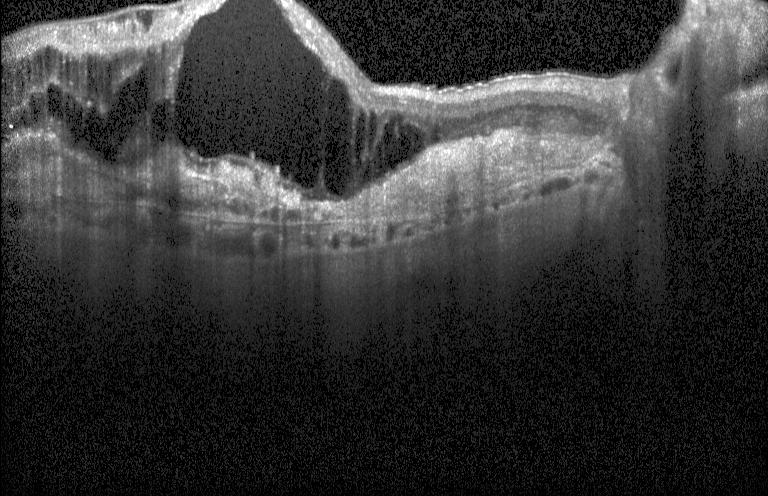

Optical coherence tomography scan. Acquired on a Heidelberg Spectralis. Spectral-domain optical coherence tomography. Macular scan
OCT finding: choroidal neovascularization (CNV).